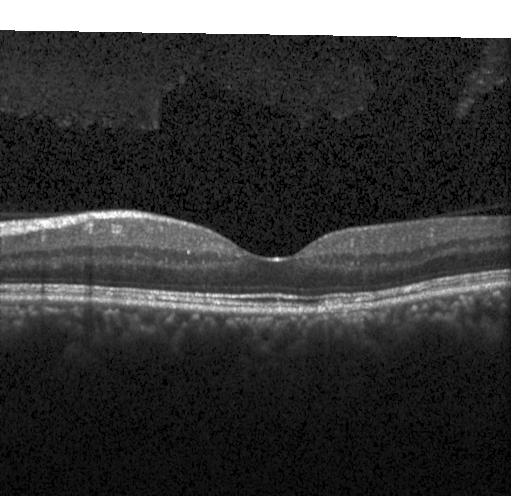

Dx: no choroidal neovascularization, no diabetic macular edema, and no drusen.